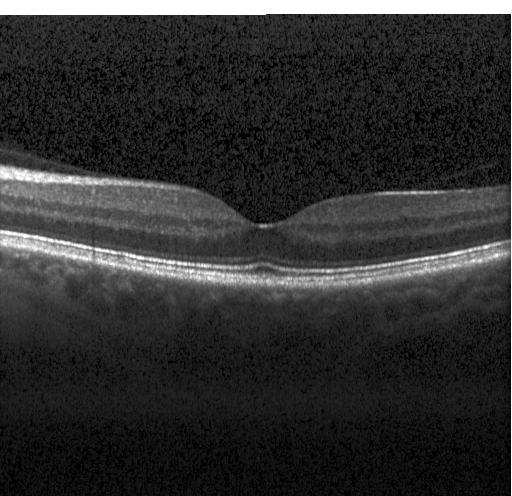

Diagnosis: neither CNV, DME, nor drusen.